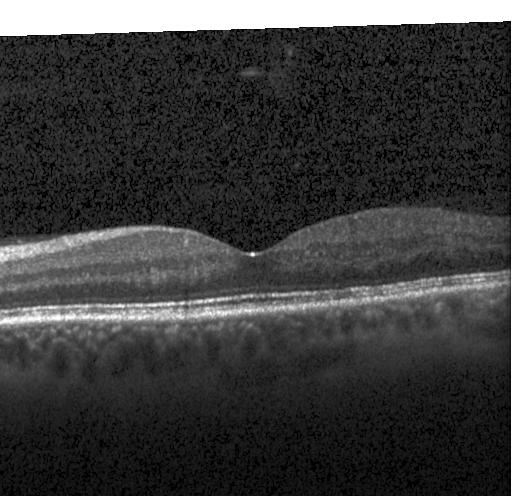

Spectral-domain optical coherence tomography; instrument: Heidelberg Spectralis; OCT line scan — OCT finding: no evidence of choroidal neovascularization, diabetic macular edema, or drusen.